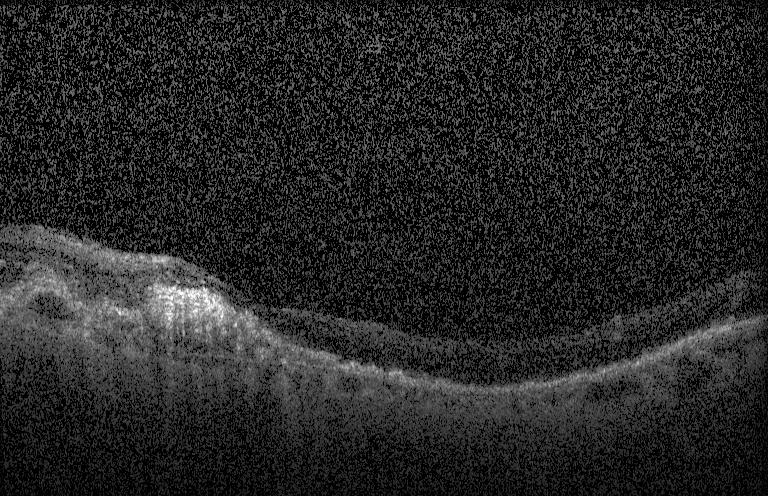

Spectral-domain OCT, optical coherence tomography scan, acquired on a Heidelberg Spectralis. Impression: CNV.